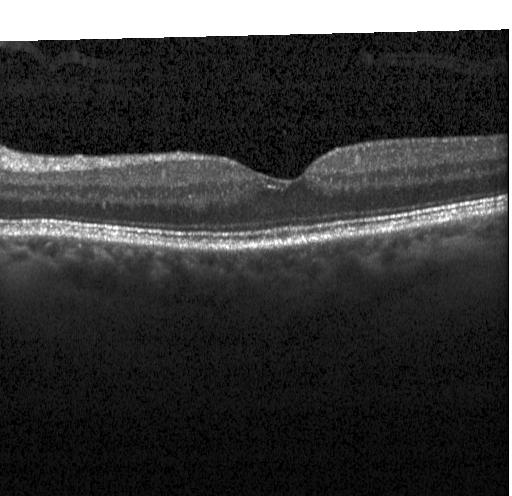

Dx: no evidence of CNV, DME, or drusen.